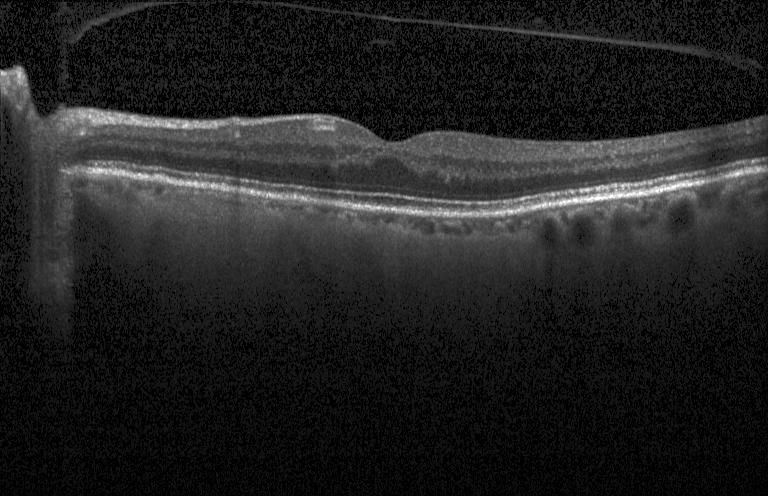
Macular OCT demonstrating no evidence of CNV, DME, or drusen.